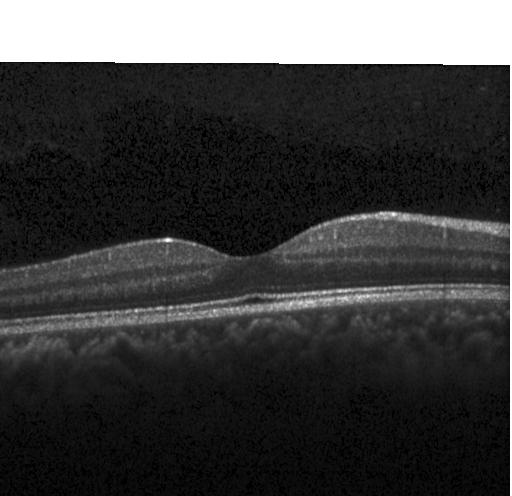
Retinal OCT cross-section — No CNV, no DME, and no drusen.